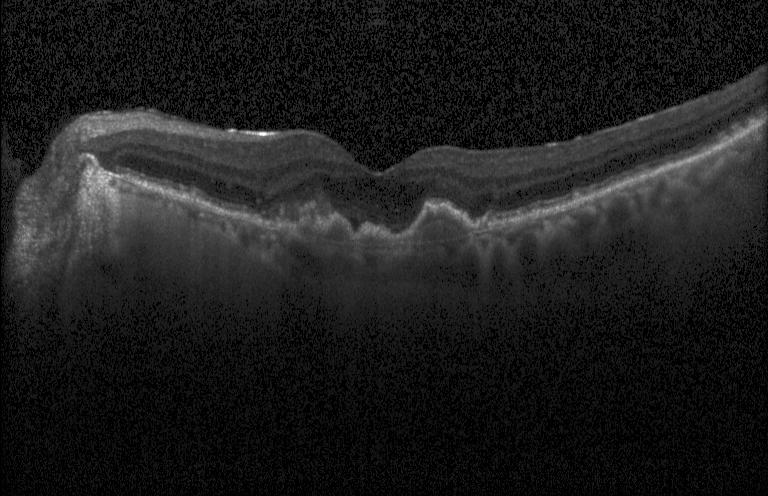

Retinal OCT B-scan.
Impression: a choroidal neovascular membrane.